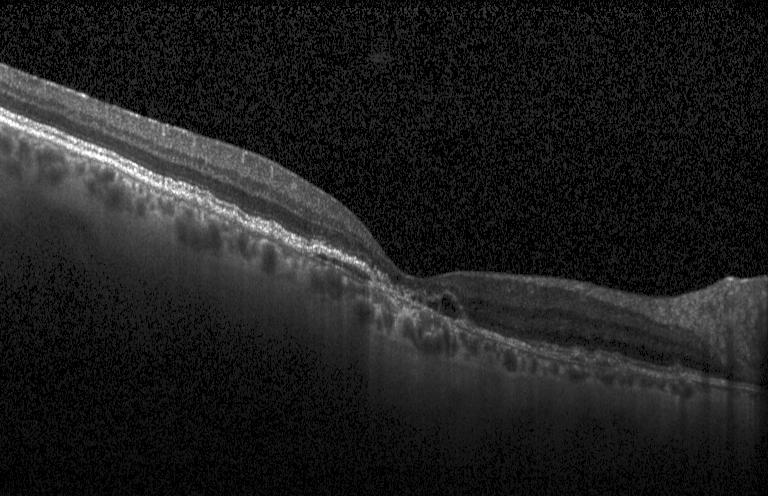
Optical coherence tomography scan — Macular OCT: a choroidal neovascular membrane.